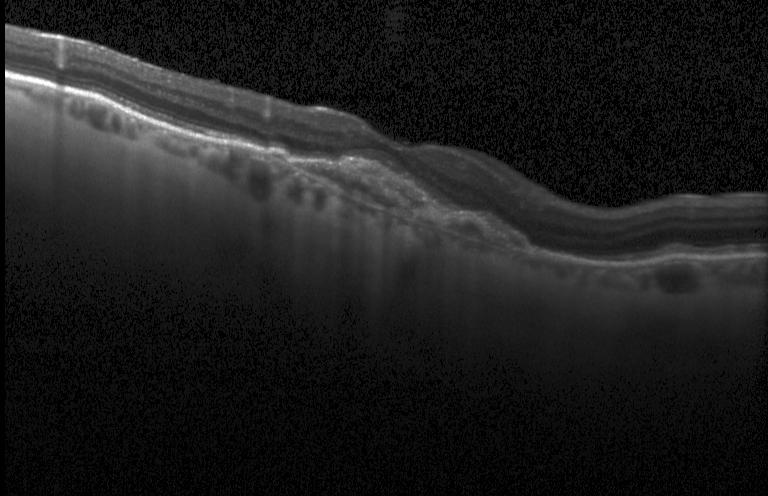

OCT B-scan.
Choroidal neovascularization.